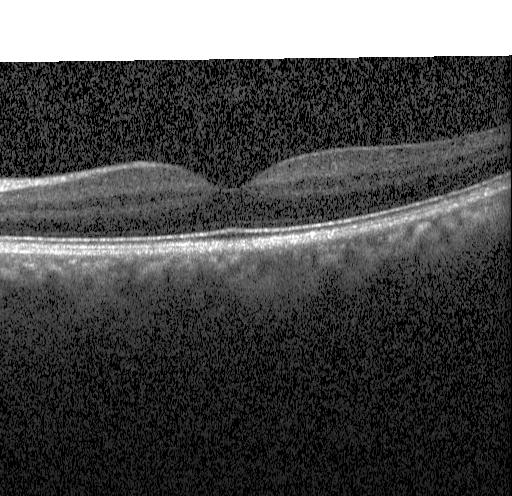

Heidelberg Spectralis; SD-OCT; centered on the fovea; OCT B-scan. Diagnosis: no choroidal neovascularization, no diabetic macular edema, and no drusen.